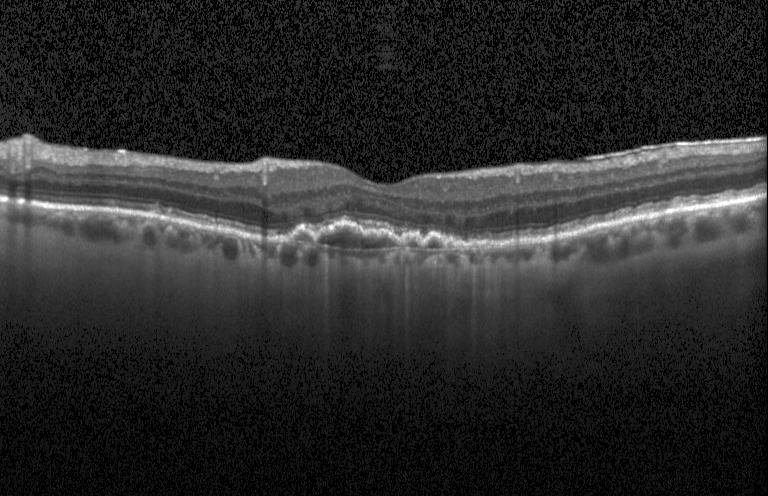 Horizontal scan through the fovea, Heidelberg Spectralis, optical coherence tomography B-scan, spectral-domain optical coherence tomography. This B-scan demonstrates a choroidal neovascular membrane.